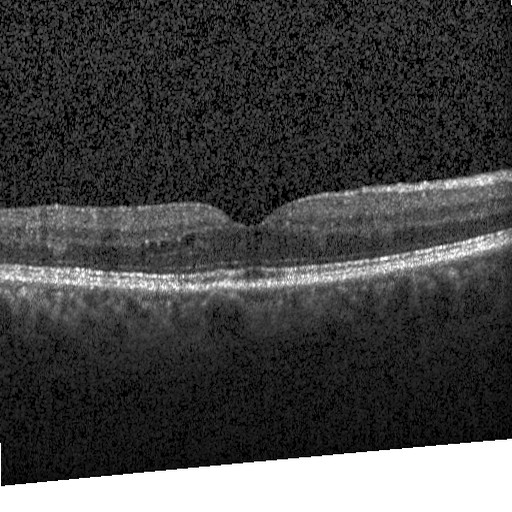 Spectral-domain optical coherence tomography; retinal OCT B-scan.
This B-scan demonstrates DME.